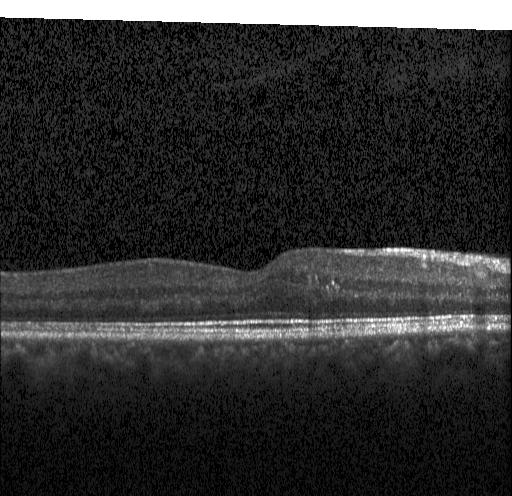 Retinal OCT B-scan · spectral-domain optical coherence tomography · instrument: Heidelberg Spectralis · fovea-centered.
No choroidal neovascularization, no diabetic macular edema, and no drusen.